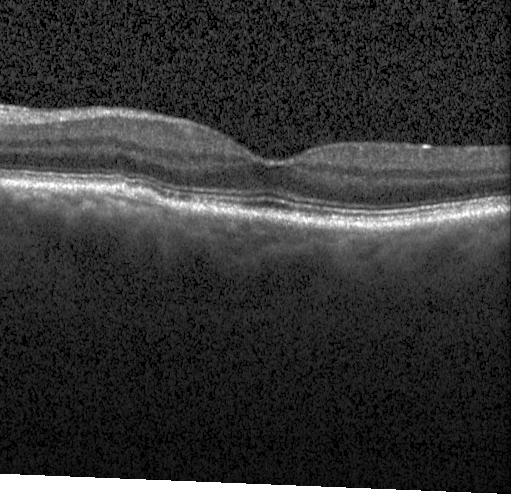 Retinal OCT cross-section, SD-OCT.
Impression: drusen.